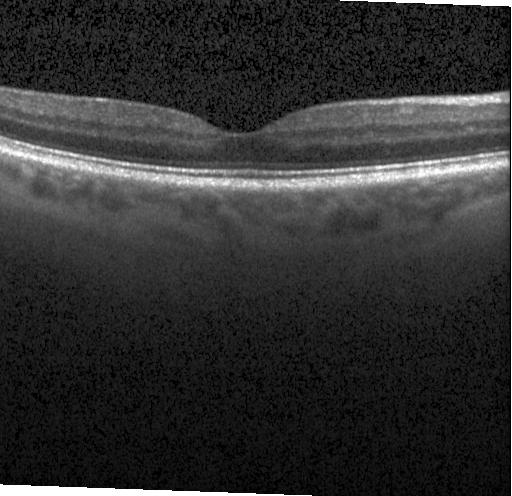

Dx: neither choroidal neovascularization, diabetic macular edema, nor drusen.